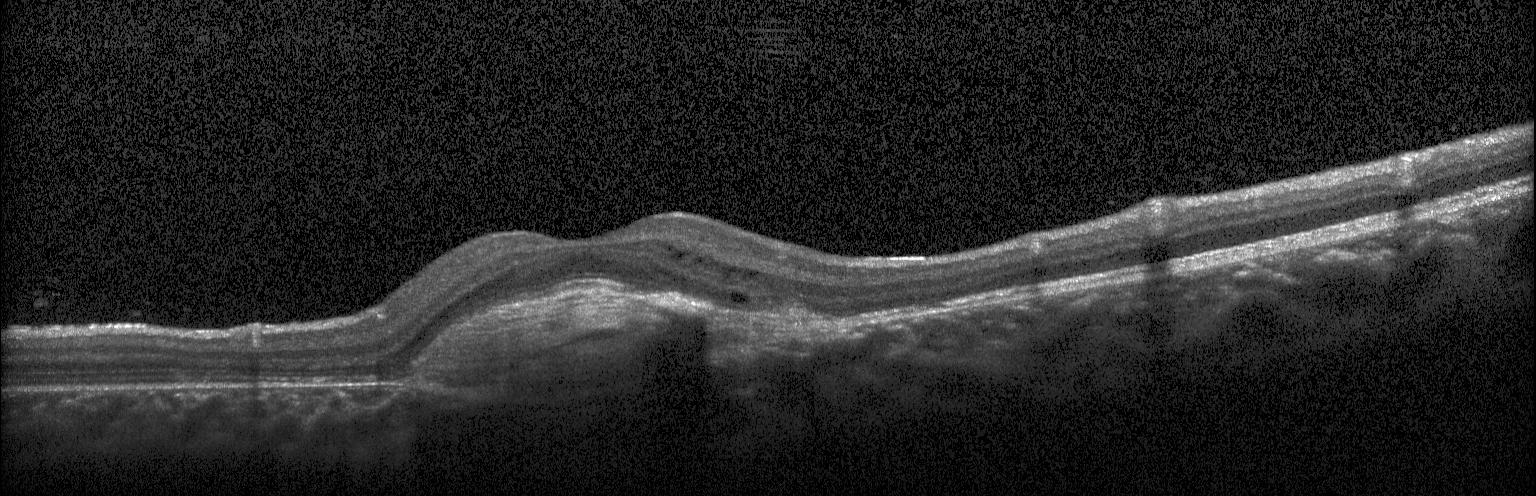 Spectral-domain OCT, instrument: Heidelberg Spectralis, optical coherence tomography scan. Macular OCT: CNV.